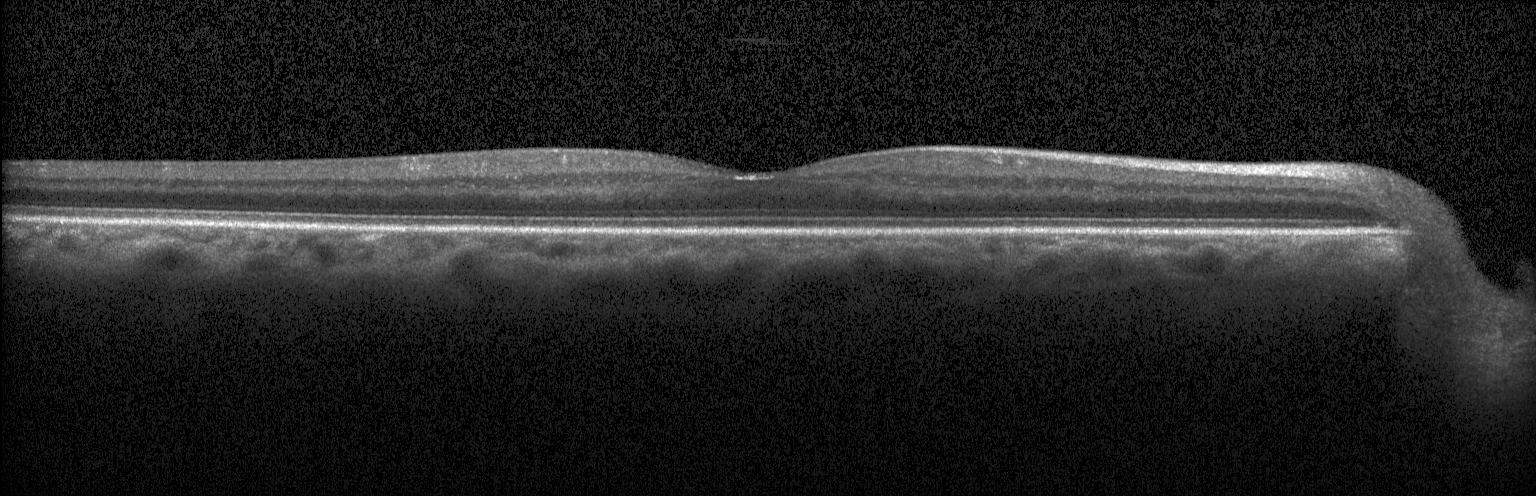
Spectral-domain OCT · horizontal scan through the fovea · optical coherence tomography B-scan · acquired on a Heidelberg Spectralis — Diagnosis: no CNV, no DME, and no drusen.